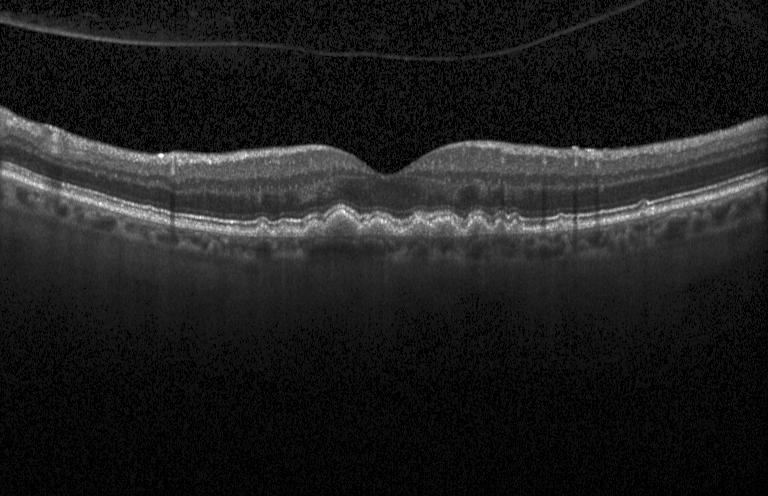
OCT B-scan, centered on the fovea, Heidelberg Spectralis OCT system. Drusen.